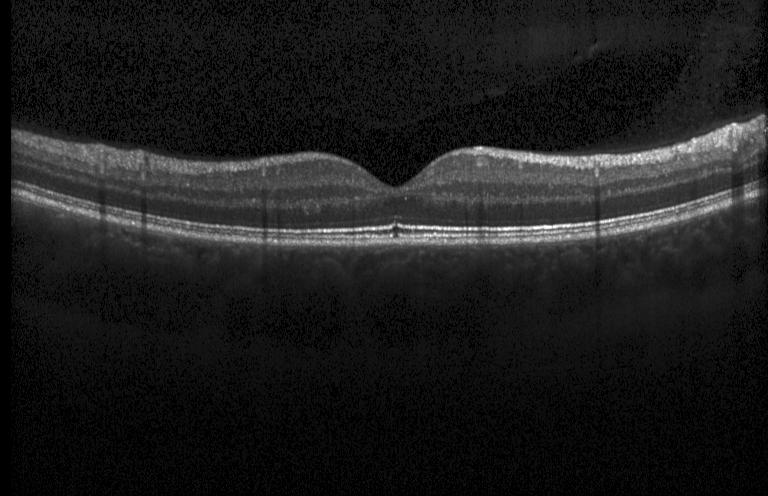

OCT B-scan. Spectral-domain optical coherence tomography. Macular scan
Assessment: no evidence of choroidal neovascularization, diabetic macular edema, or drusen.